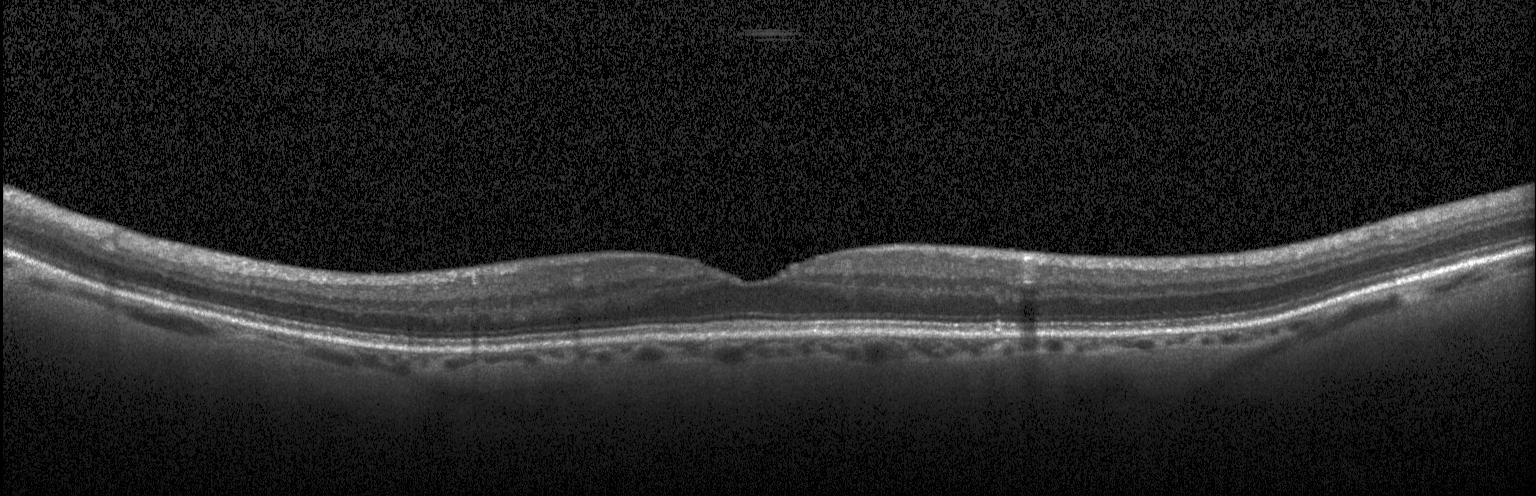 Finding: no CNV, no DME, and no drusen.